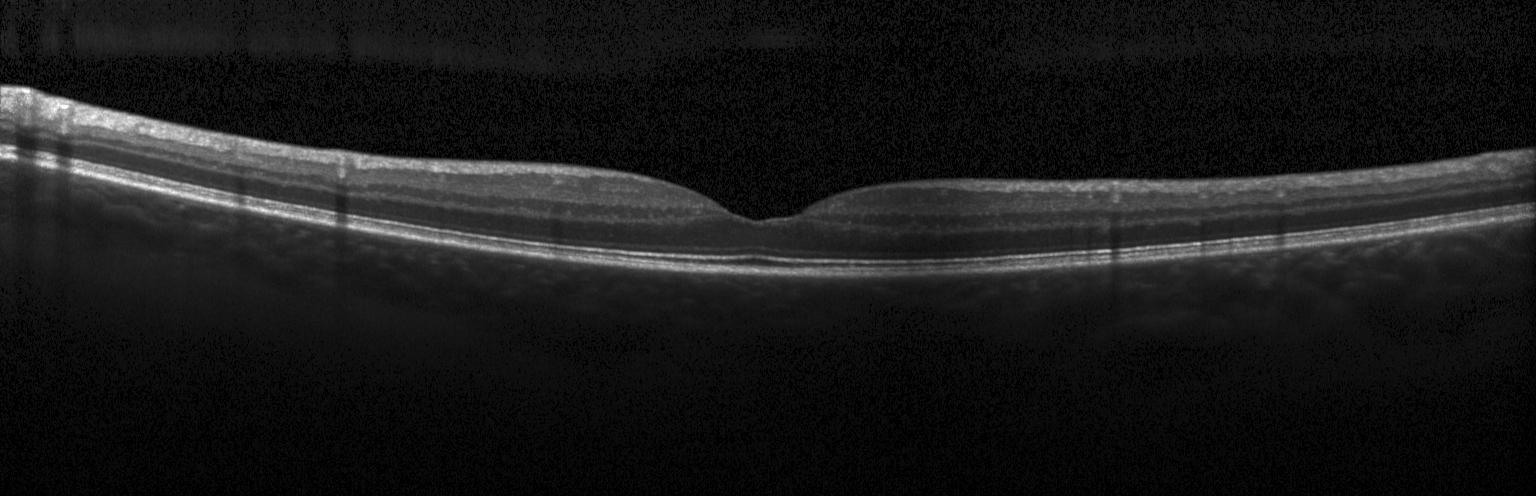 Optical coherence tomography scan; Heidelberg Spectralis; fovea-centered; SD-OCT
This B-scan demonstrates no choroidal neovascularization, diabetic macular edema, or drusen.